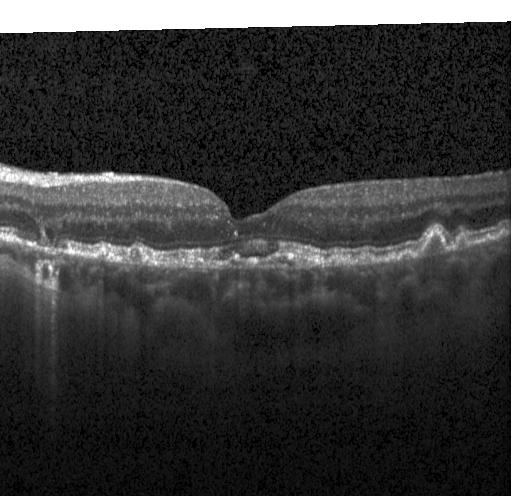 Assessment: a choroidal neovascular membrane.